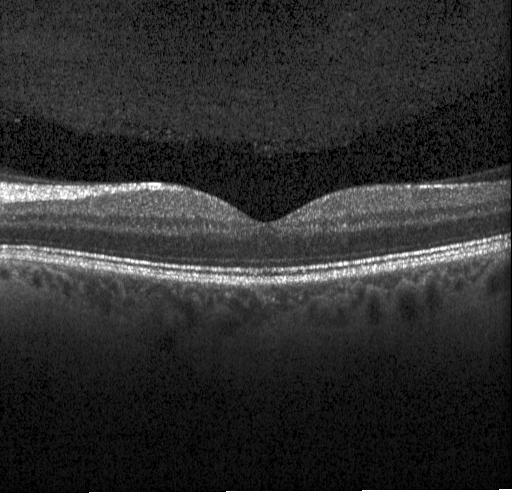 No CNV, DME, or drusen.